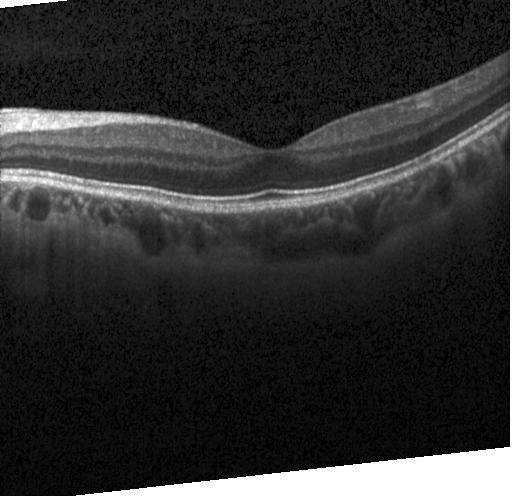 Macular OCT: neither CNV, DME, nor drusen.